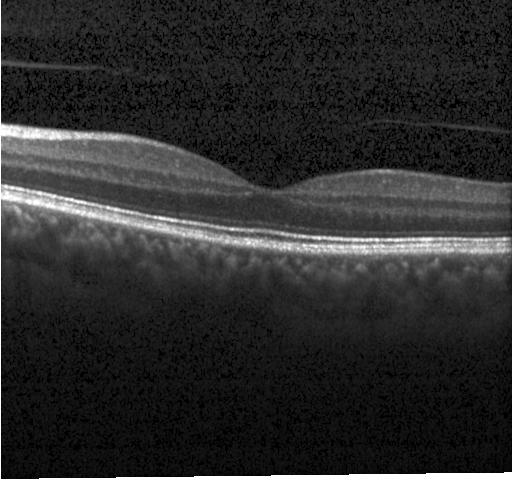

Retinal OCT cross-section showing no CNV, DME, or drusen.